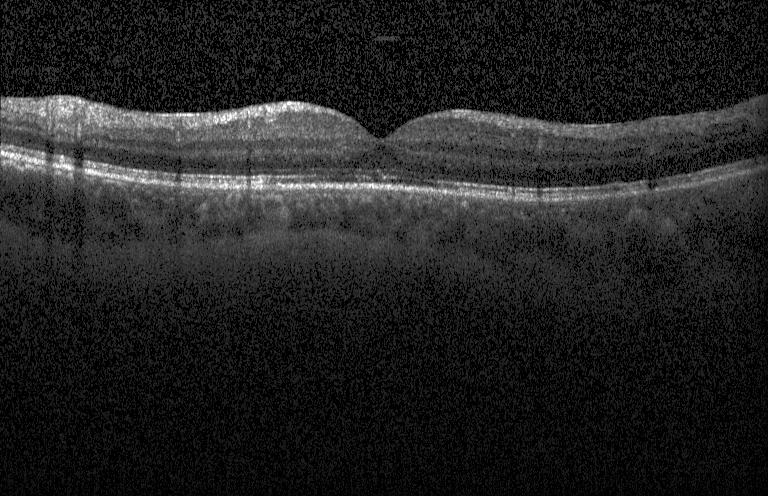 Macular OCT: neither choroidal neovascularization, diabetic macular edema, nor drusen.